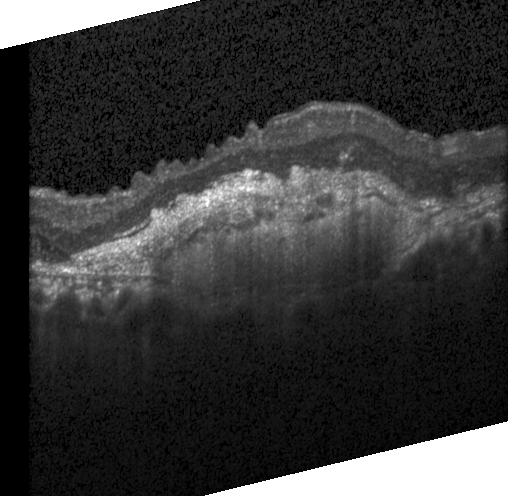

Retinal OCT cross-section. Fovea-centered — Diagnosis: a choroidal neovascular membrane.